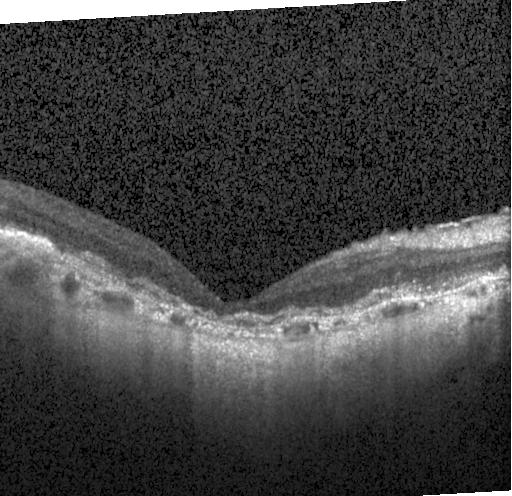
Fovea-centered; retinal OCT cross-section; acquired on a Heidelberg Spectralis. A choroidal neovascular membrane.